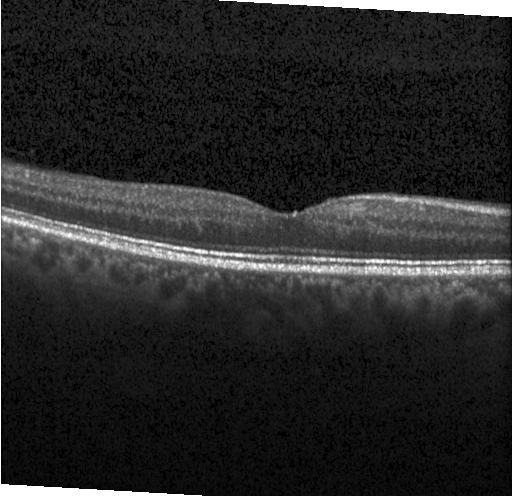 OCT B-scan. Heidelberg Spectralis. Spectral-domain optical coherence tomography. Horizontal scan through the fovea.
The scan shows neither choroidal neovascularization, diabetic macular edema, nor drusen.